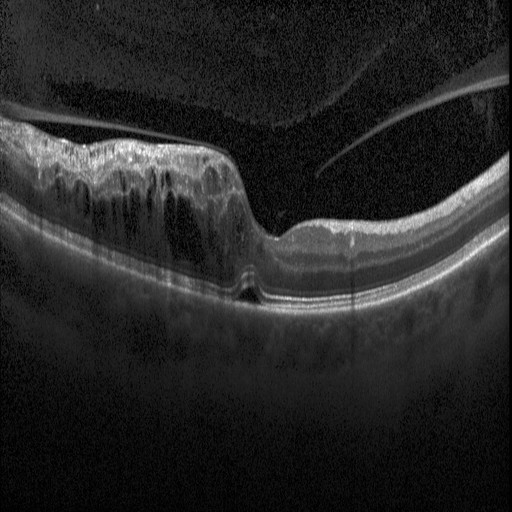 Optical coherence tomography B-scan — Diabetic macular edema (DME).